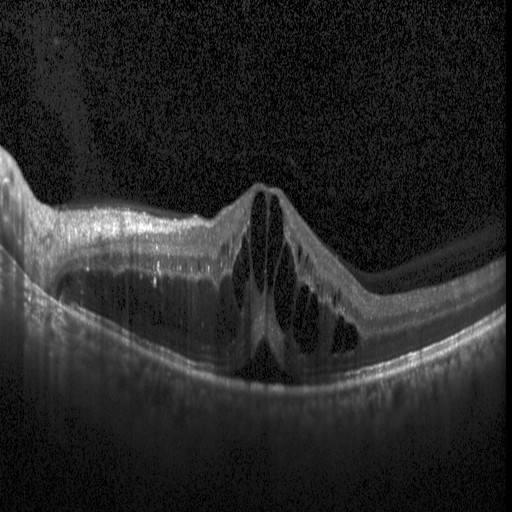

Retinal OCT cross-section. Macular scan. Spectral-domain OCT — Assessment: diabetic macular edema (DME).